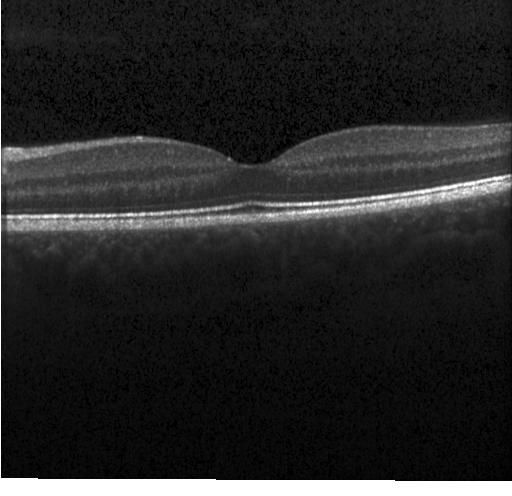 The scan shows no CNV, DME, or drusen.